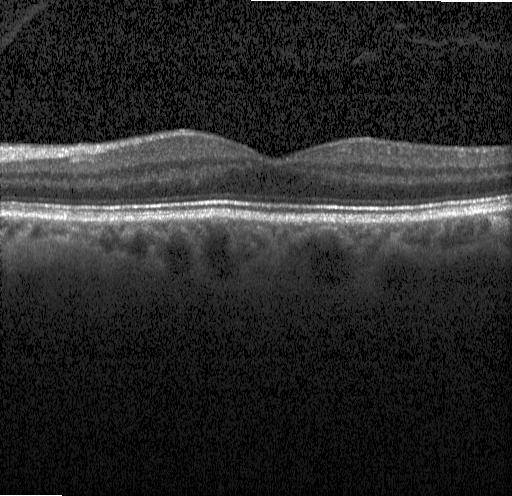

Optical coherence tomography scan; macular scan; Heidelberg Spectralis OCT system; SD-OCT — Finding: neither CNV, DME, nor drusen.